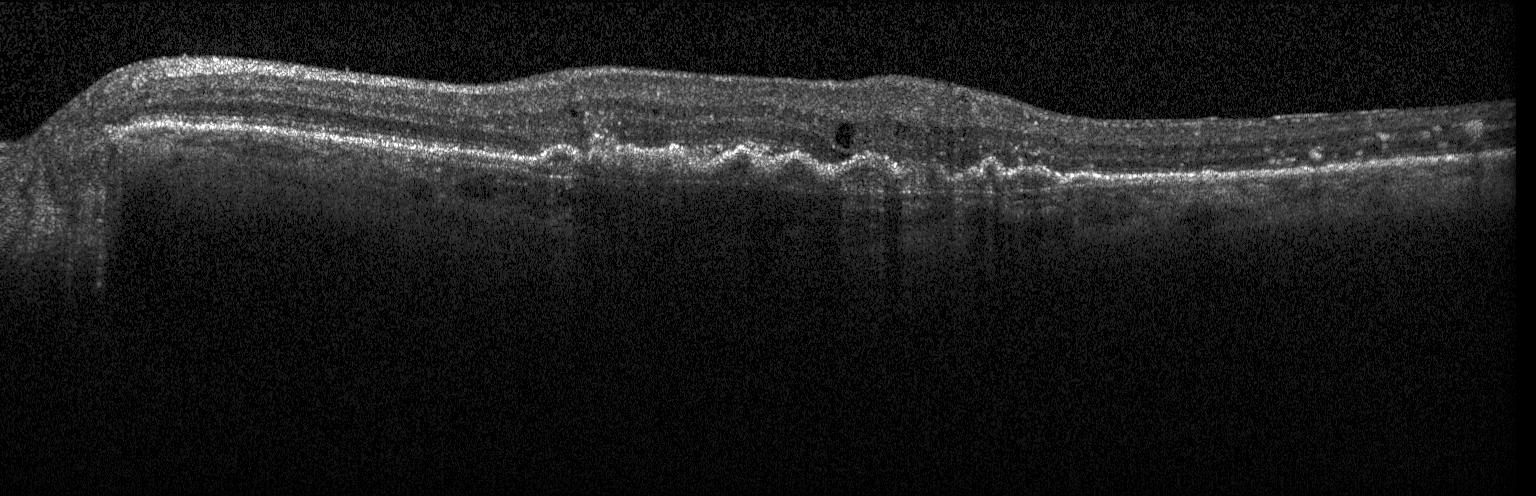
Dx: choroidal neovascularization.